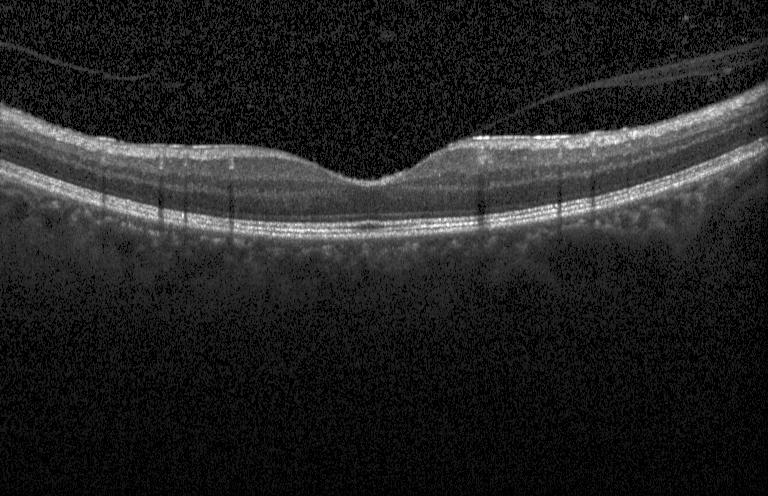
Diagnosis: no evidence of choroidal neovascularization, diabetic macular edema, or drusen.